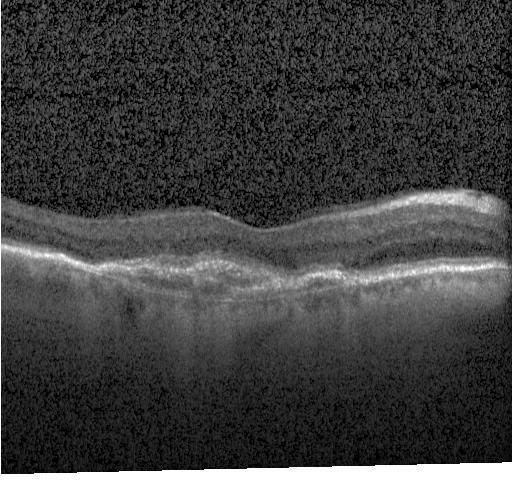
Optical coherence tomography B-scan; horizontal scan through the fovea — Impression: a choroidal neovascular membrane.